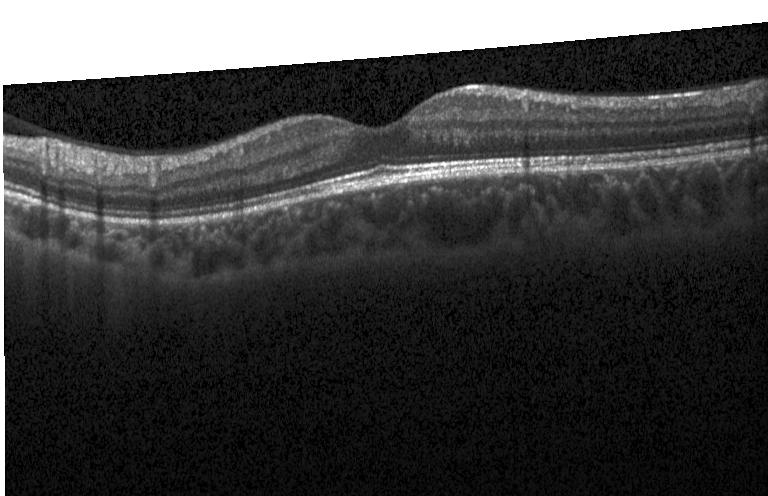

Macular scan · OCT B-scan · Heidelberg Spectralis — Assessment: no choroidal neovascularization, no diabetic macular edema, and no drusen.